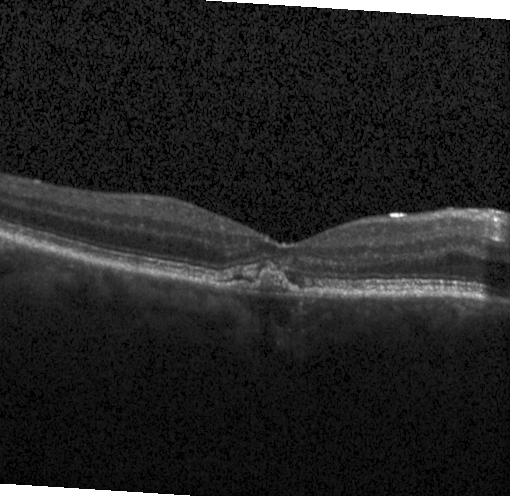 OCT B-scan, spectral-domain optical coherence tomography, horizontal scan through the fovea, Heidelberg Spectralis.
The scan shows CNV.